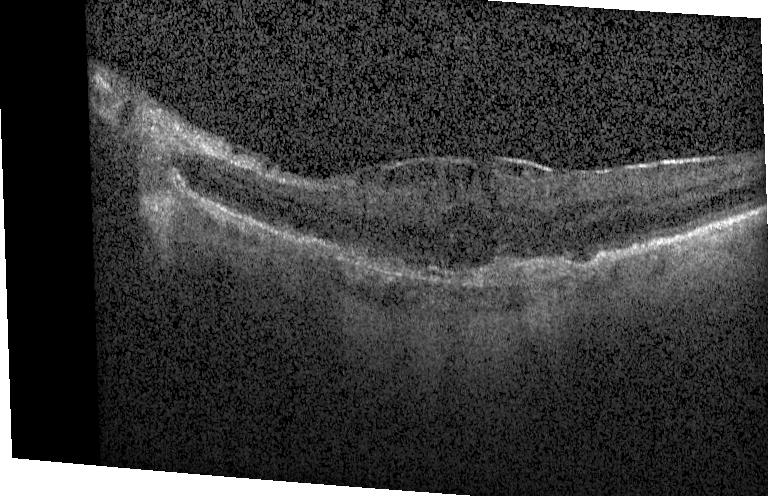

Horizontal scan through the fovea, optical coherence tomography B-scan.
This B-scan demonstrates a choroidal neovascular membrane.